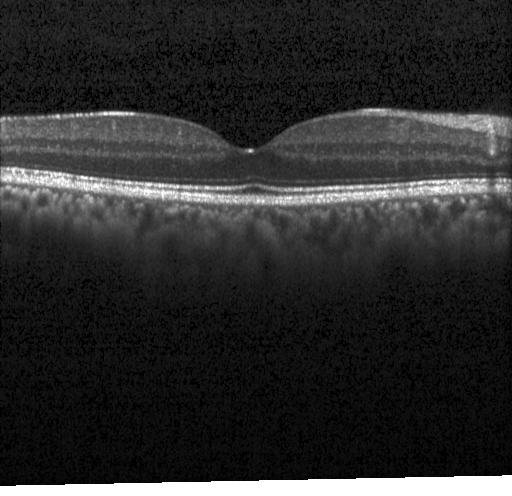
OCT B-scan.
Diagnosis: no choroidal neovascularization, diabetic macular edema, or drusen.